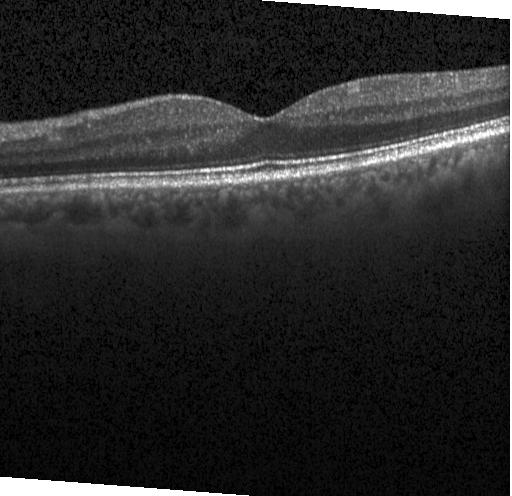

Diagnosis: no choroidal neovascularization, no diabetic macular edema, and no drusen.